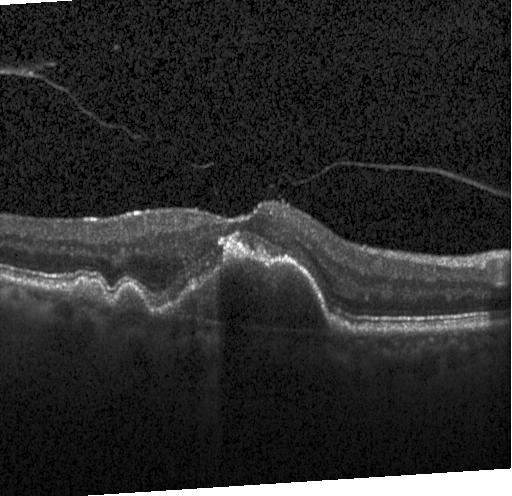

Diagnosis: CNV.